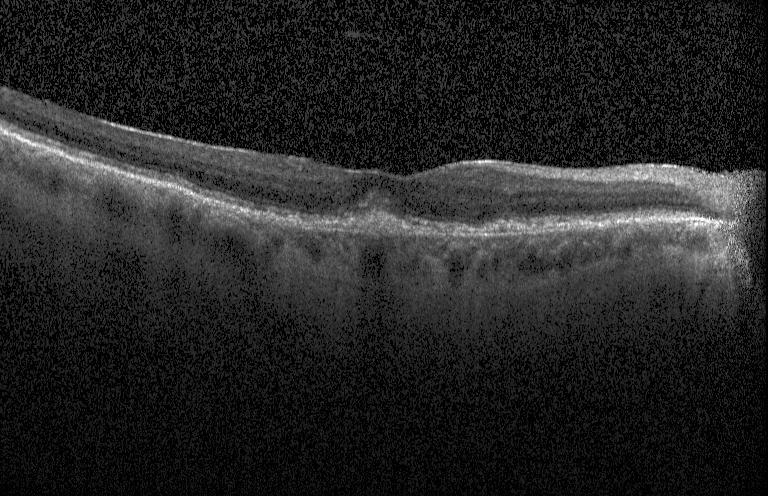
Optical coherence tomography B-scan · acquired on a Heidelberg Spectralis · spectral-domain OCT · macular scan. This B-scan demonstrates choroidal neovascularization (CNV).